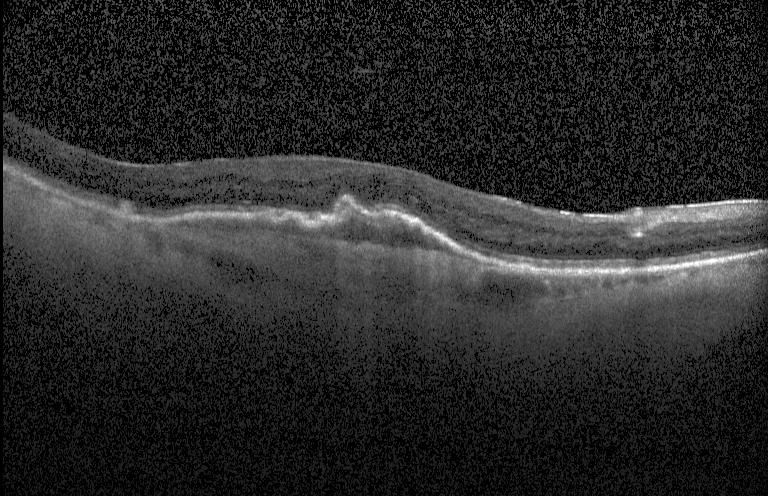
Spectral-domain OCT B-scan: CNV.